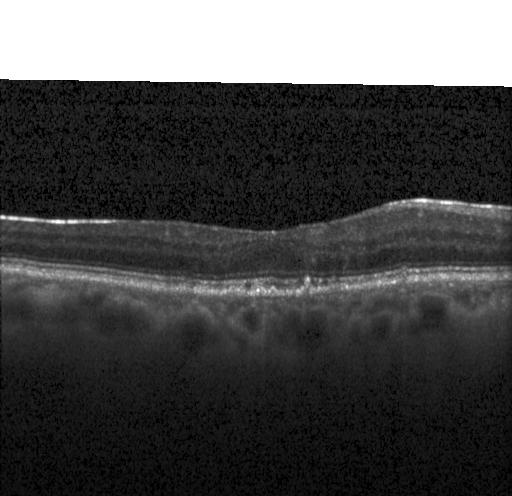

Heidelberg Spectralis. Through the macula. Optical coherence tomography scan. Spectral-domain optical coherence tomography.
Impression: multiple drusen.